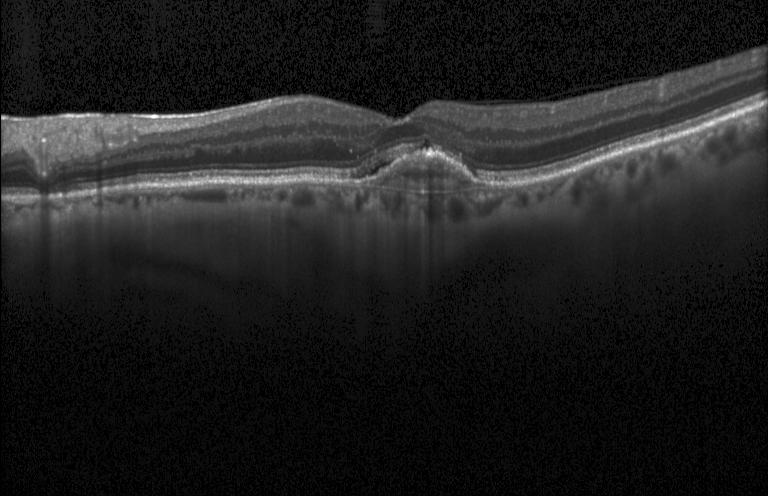

OCT line scan.
Diagnosis: a choroidal neovascular membrane.